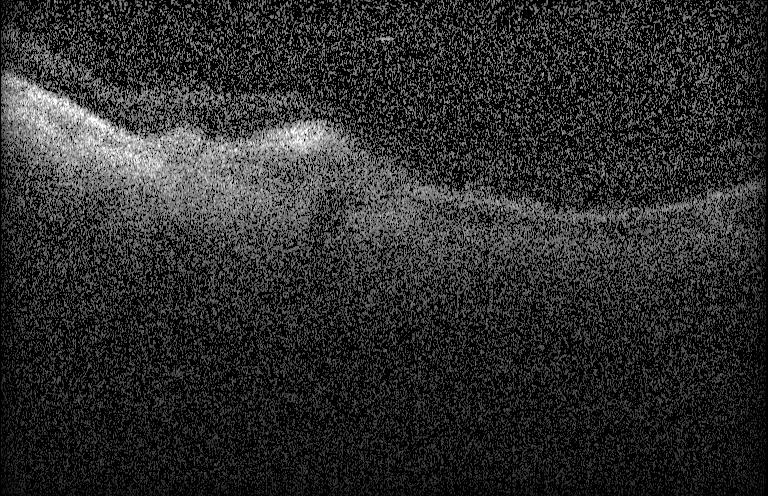

Impression: choroidal neovascularization.